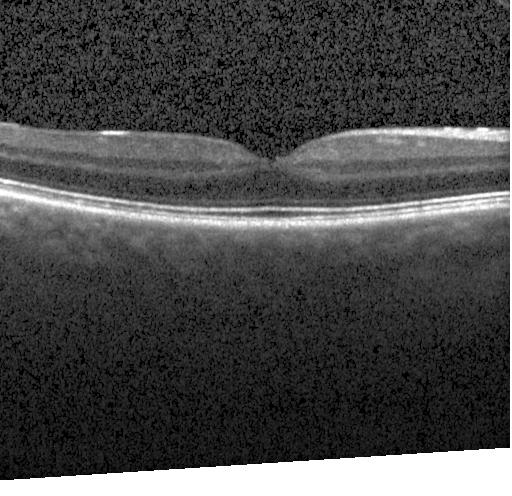 Spectral-domain OCT; OCT B-scan — This B-scan demonstrates neither CNV, DME, nor drusen.